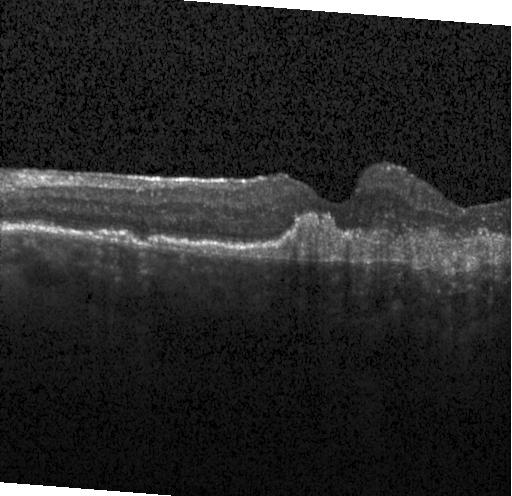

Instrument: Heidelberg Spectralis, fovea-centered, retinal OCT B-scan. A choroidal neovascular membrane.